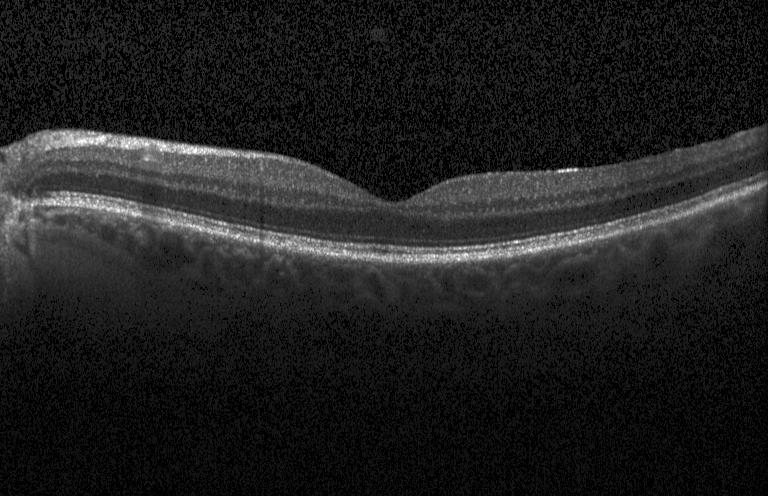 Macular scan. Spectral-domain OCT. OCT B-scan. Instrument: Heidelberg Spectralis. Impression: no choroidal neovascularization, diabetic macular edema, or drusen.